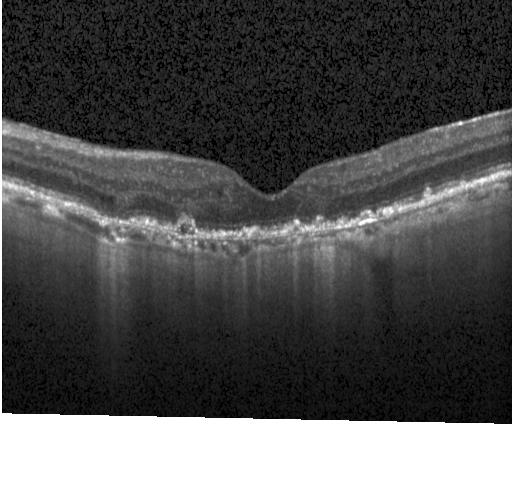 This B-scan demonstrates choroidal neovascularization (CNV).